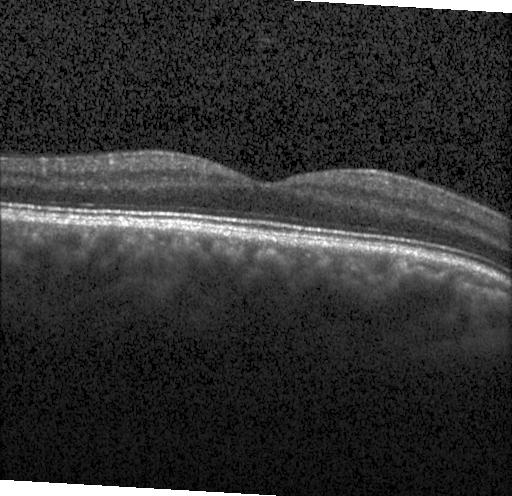

This B-scan demonstrates no evidence of choroidal neovascularization, diabetic macular edema, or drusen.